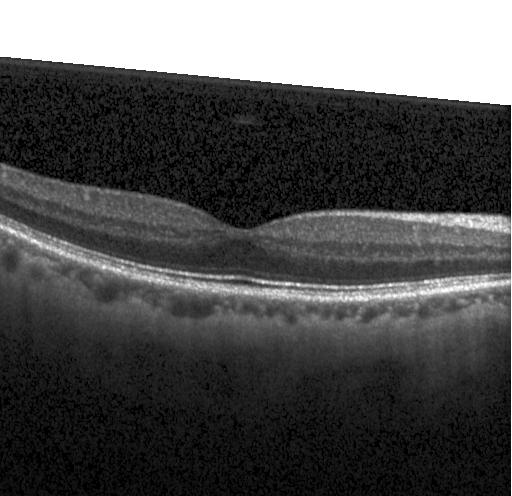
Retinal OCT cross-section. Diagnosis: no choroidal neovascularization, no diabetic macular edema, and no drusen.